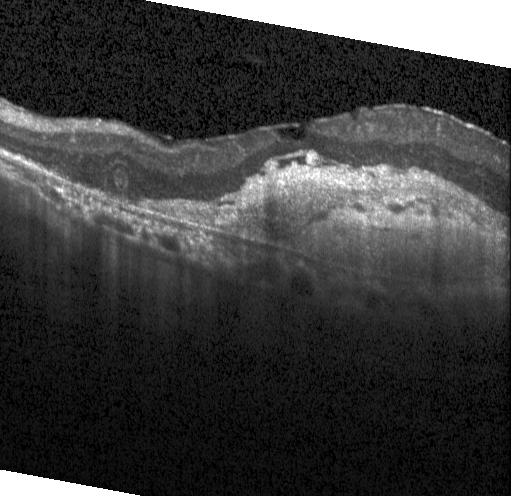 Impression: choroidal neovascularization.